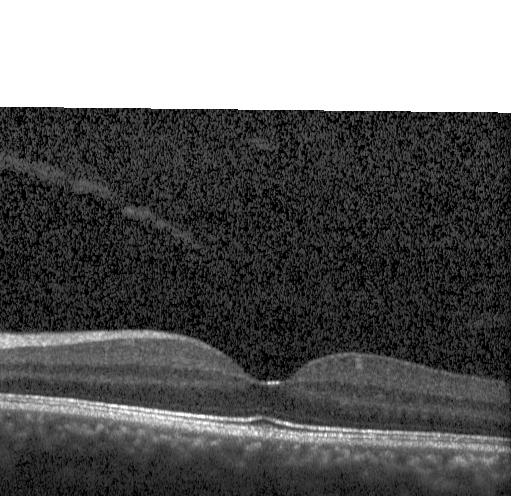
The scan shows no choroidal neovascularization, diabetic macular edema, or drusen.